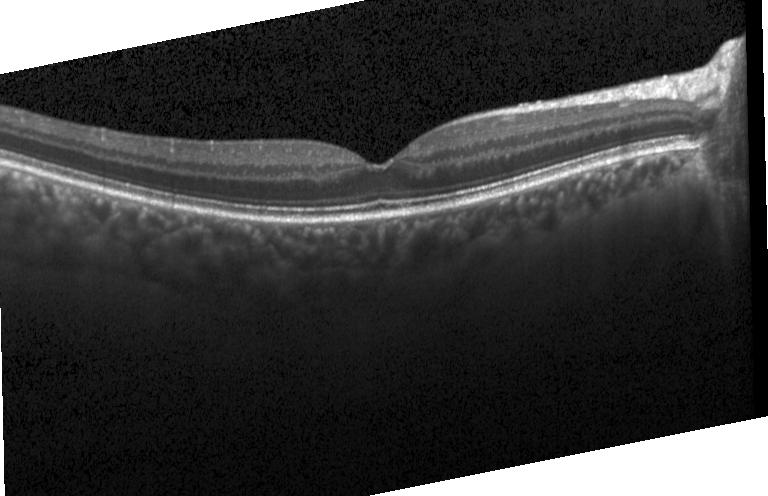
Impression: no evidence of choroidal neovascularization, diabetic macular edema, or drusen.